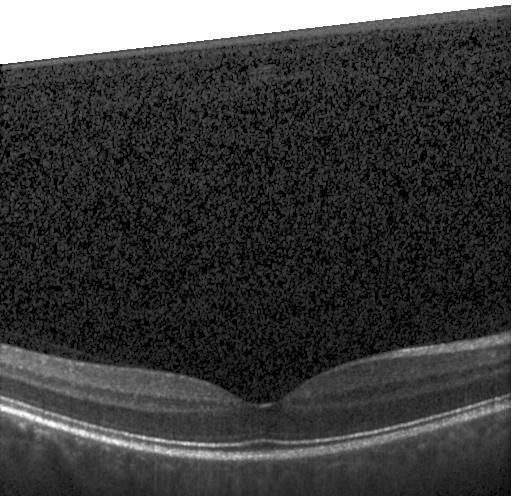 Retinal OCT B-scan · spectral-domain optical coherence tomography
No evidence of choroidal neovascularization, diabetic macular edema, or drusen.